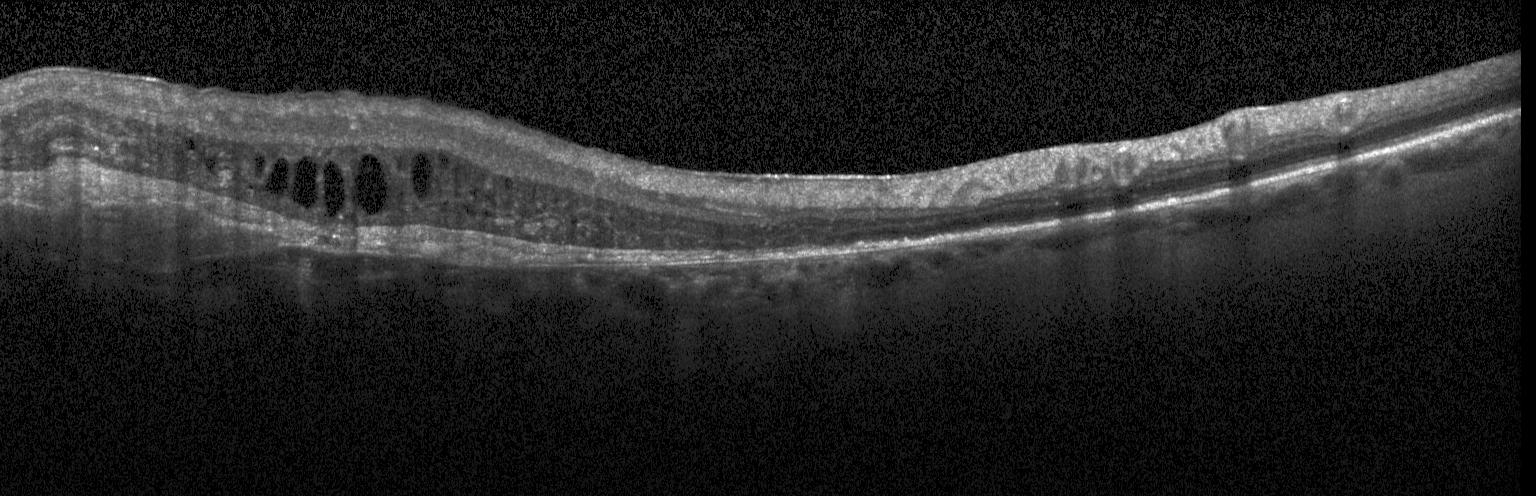 OCT B-scan. This B-scan demonstrates CNV.